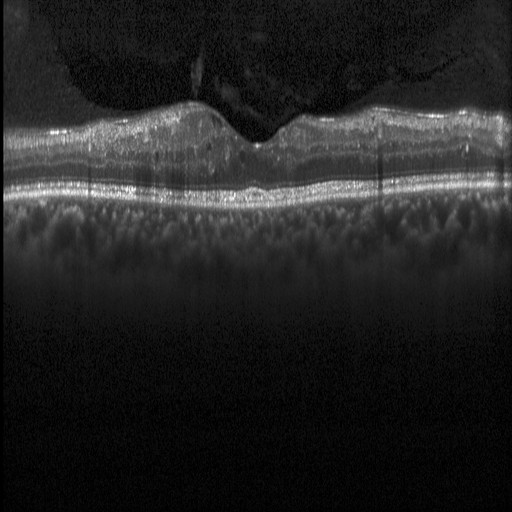 Dx: diabetic macular edema.